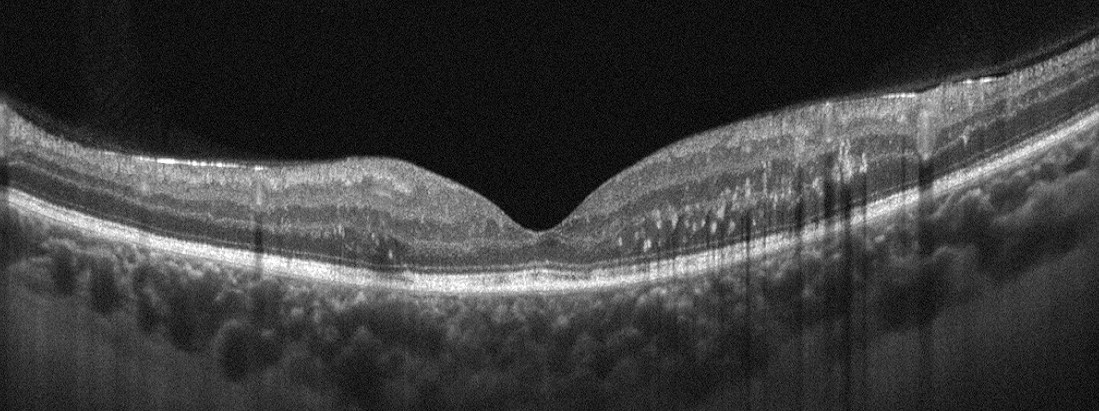

OCT B-scan showing diabetic macular edema (DME).